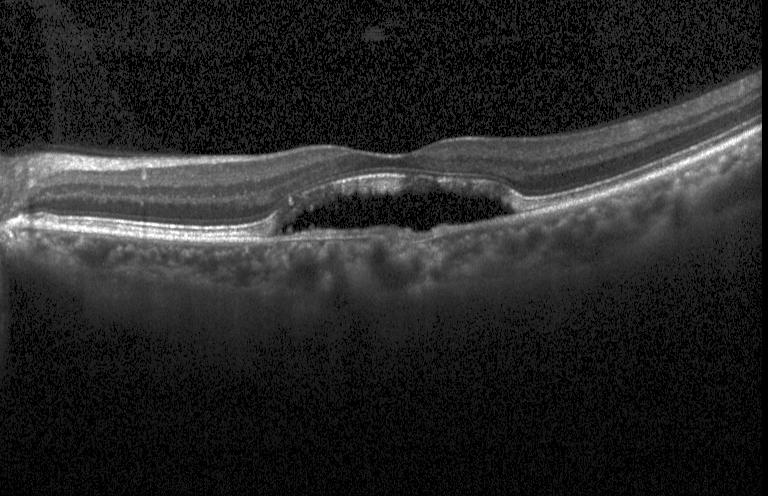 Heidelberg Spectralis; optical coherence tomography B-scan — Diagnosis: CNV.